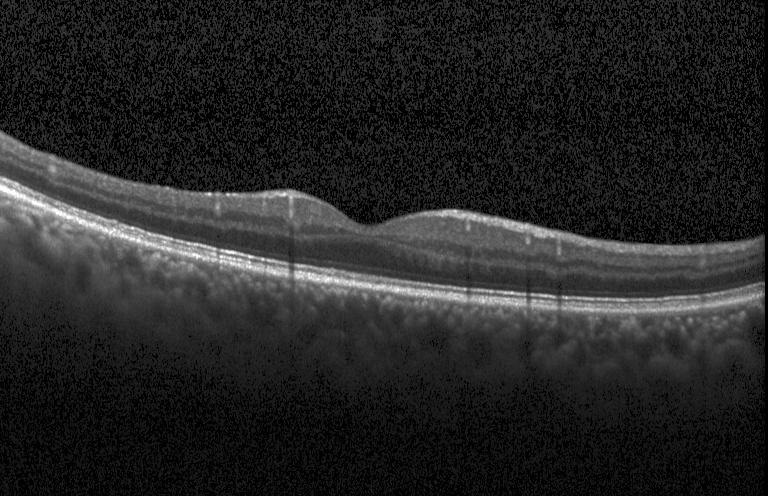

Finding: no CNV, no DME, and no drusen.